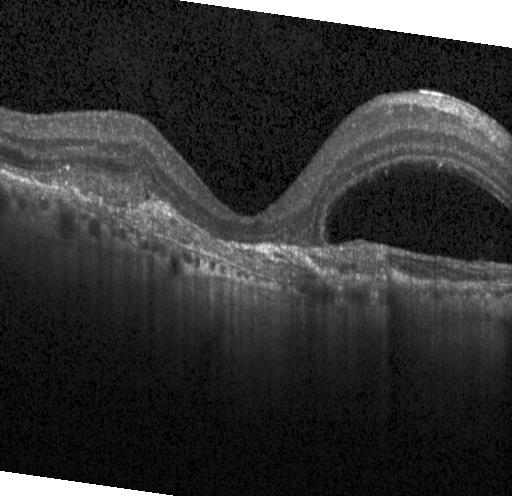
Diagnosis: choroidal neovascularization.